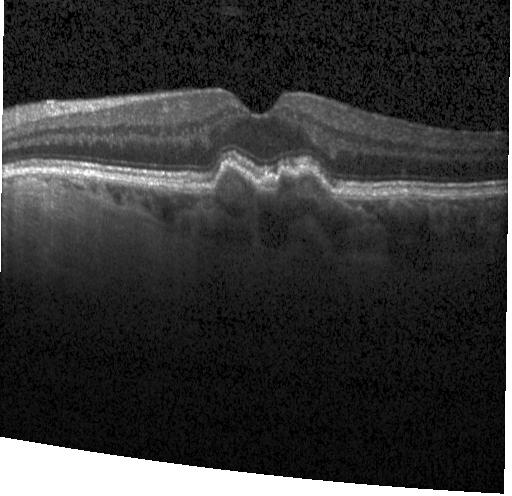 A choroidal neovascular membrane.